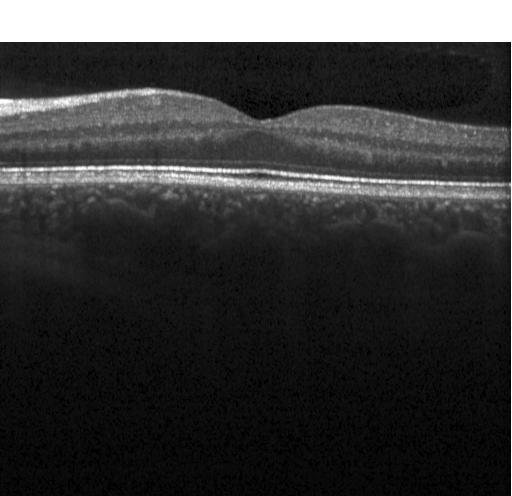 Spectral-domain optical coherence tomography · Heidelberg Spectralis · retinal OCT B-scan
The scan shows no choroidal neovascularization, diabetic macular edema, or drusen.